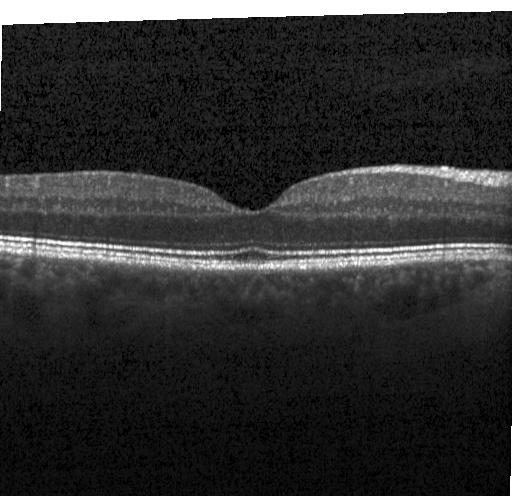
OCT B-scan, Heidelberg Spectralis.
Impression: no evidence of choroidal neovascularization, diabetic macular edema, or drusen.